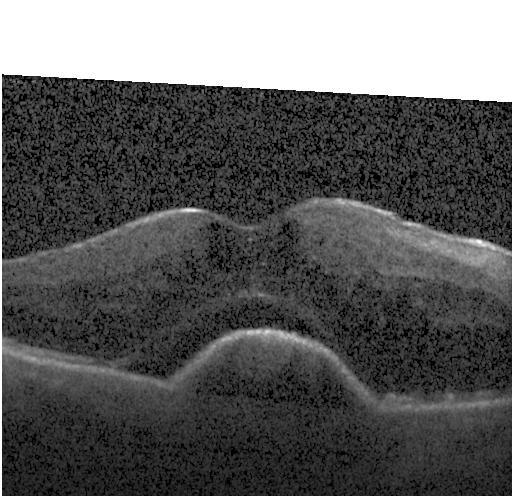

Retinal OCT B-scan, spectral-domain OCT. The scan shows a choroidal neovascular membrane.